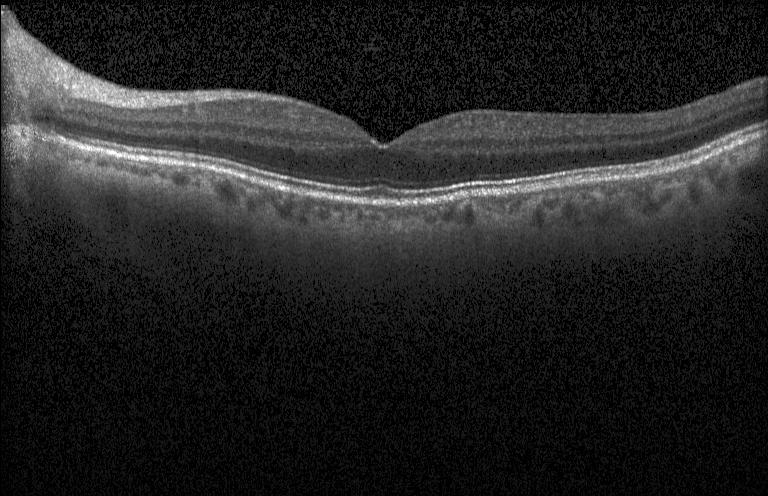 Acquired on a Heidelberg Spectralis; retinal OCT B-scan.
Dx: neither choroidal neovascularization, diabetic macular edema, nor drusen.